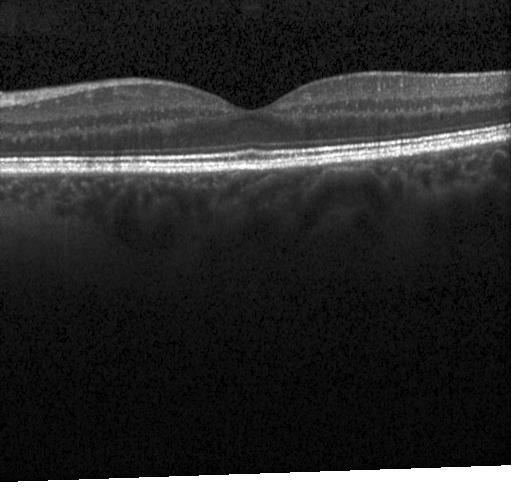 Optical coherence tomography scan
Macular OCT: no choroidal neovascularization, no diabetic macular edema, and no drusen.